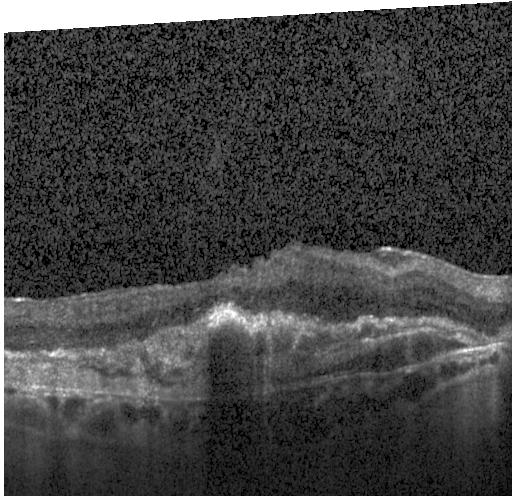
Fovea-centered. Spectral-domain OCT. OCT B-scan. Acquired on a Heidelberg Spectralis
Impression: CNV.